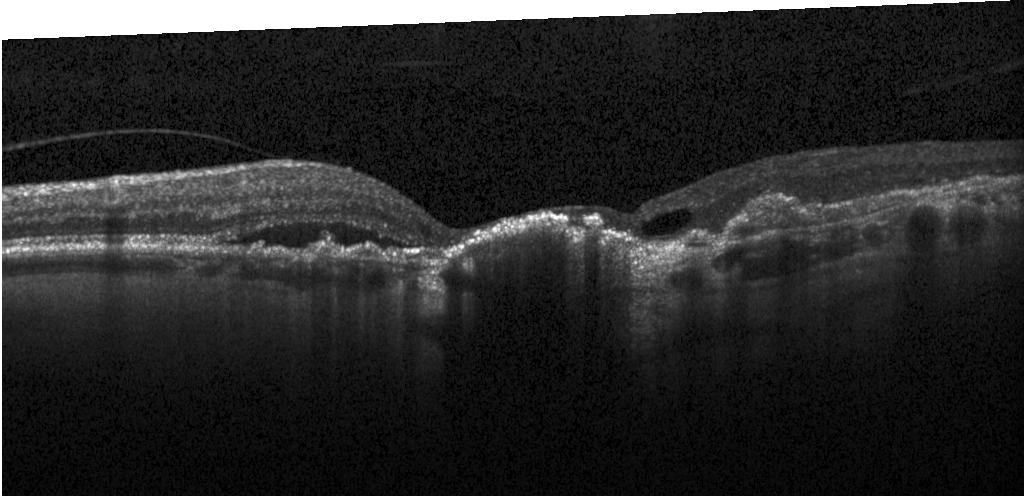

Retinal OCT B-scan, horizontal scan through the fovea — Dx: CNV.